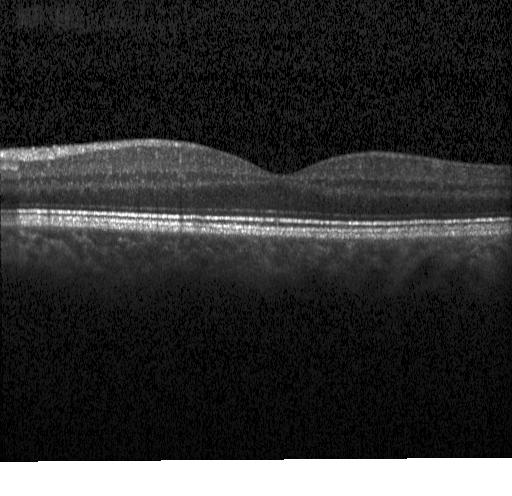
OCT B-scan. OCT finding: no choroidal neovascularization, diabetic macular edema, or drusen.